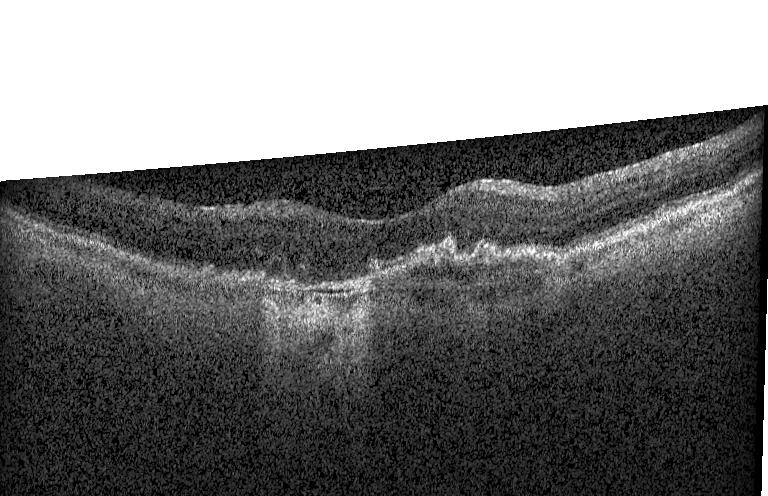
Diagnosis: CNV.